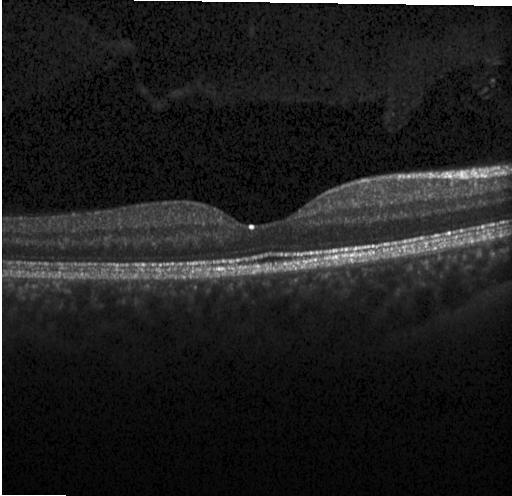
Centered on the fovea · retinal OCT cross-section. Assessment: neither CNV, DME, nor drusen.